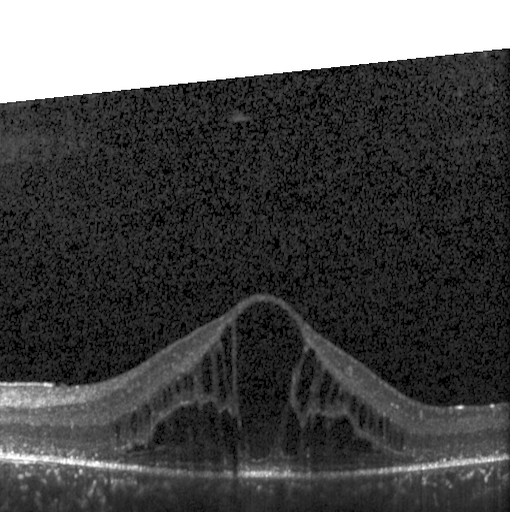

Retinal OCT cross-section; horizontal scan through the fovea; Heidelberg Spectralis OCT system
The scan shows diabetic macular edema (DME).